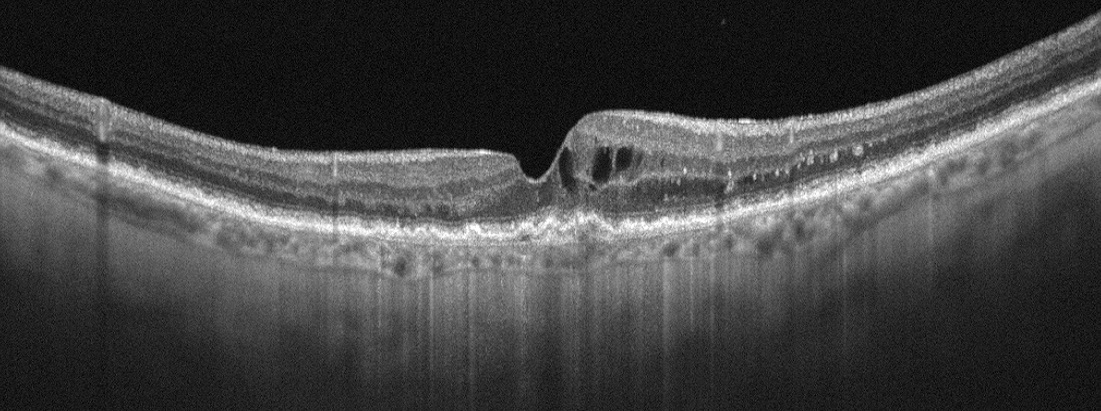 Fovea-centered · optical coherence tomography scan · Optovue Avanti RTVue XR.
The scan shows AMD.